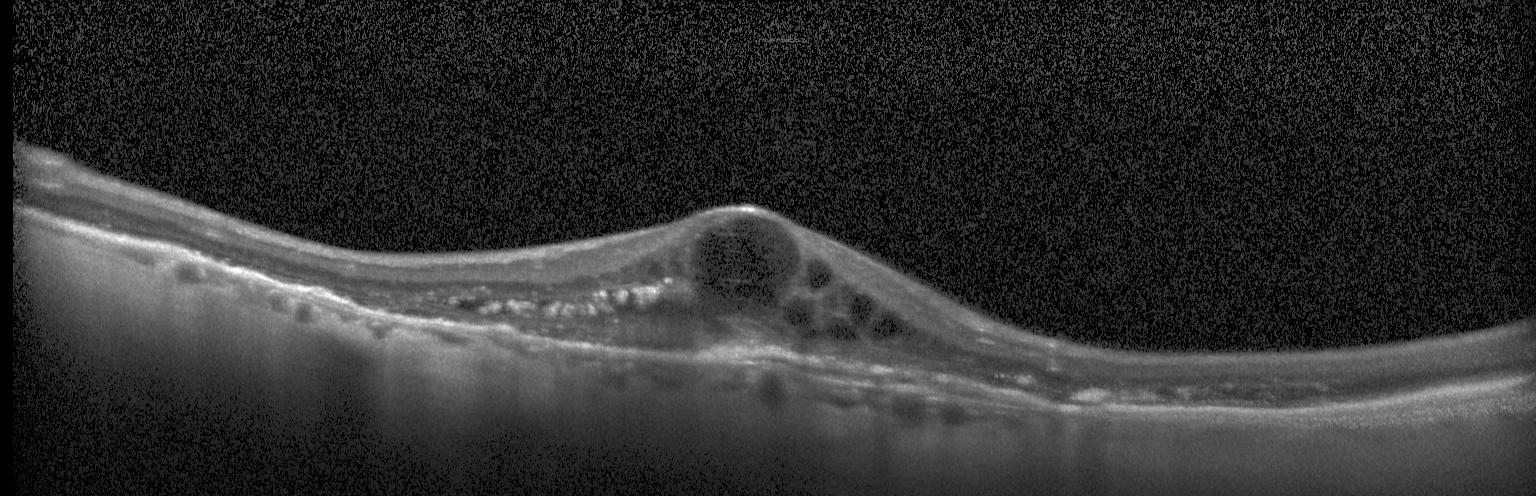
Through the macula, optical coherence tomography B-scan, spectral-domain optical coherence tomography, Heidelberg Spectralis
This B-scan demonstrates a choroidal neovascular membrane.